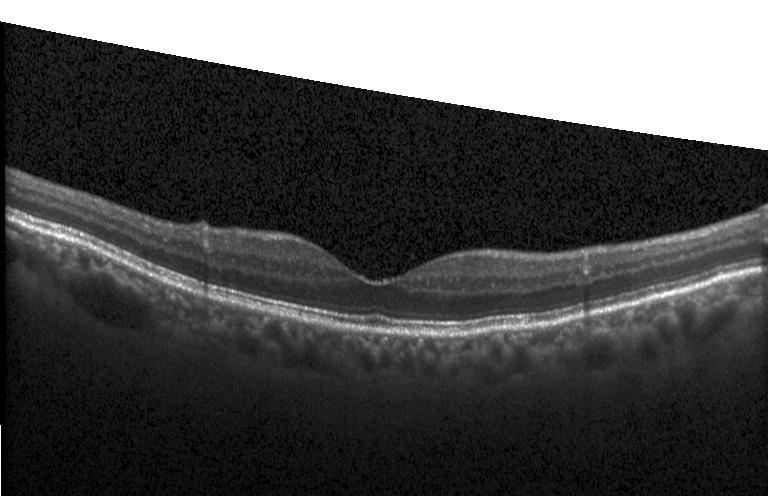
Diagnosis: neither choroidal neovascularization, diabetic macular edema, nor drusen.